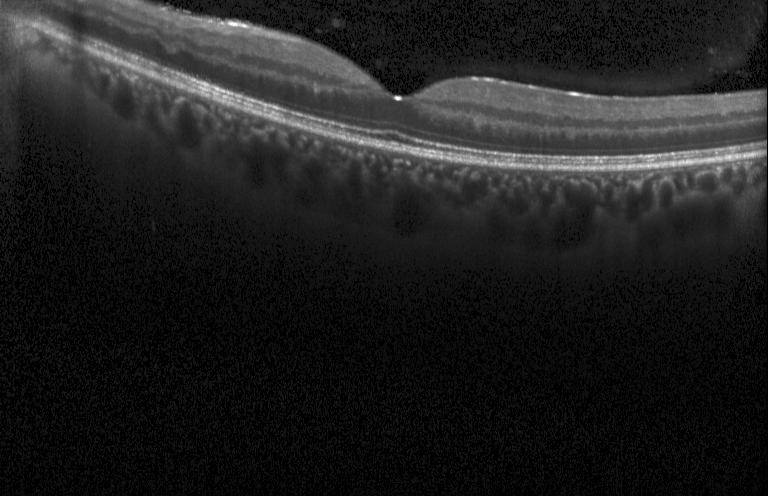
Heidelberg Spectralis. OCT B-scan.
Assessment: neither choroidal neovascularization, diabetic macular edema, nor drusen.